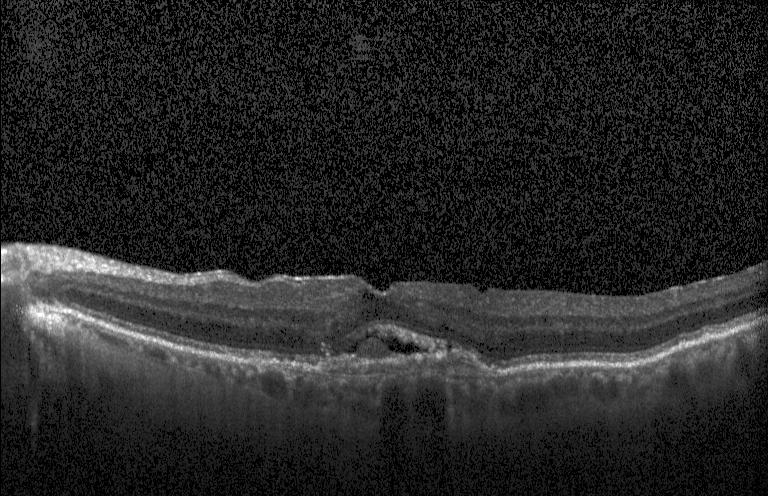 Macular OCT demonstrating CNV.